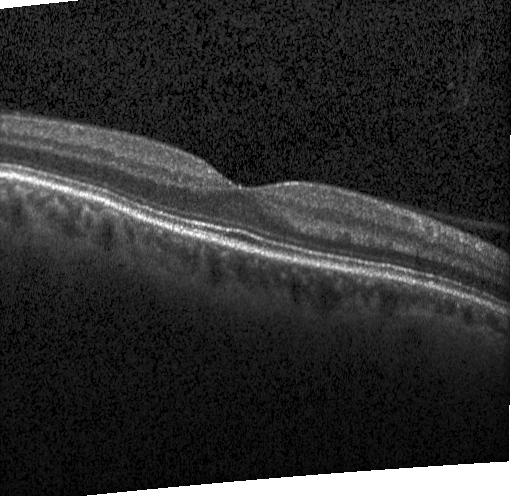

Instrument: Heidelberg Spectralis; OCT B-scan.
Macular OCT: no evidence of choroidal neovascularization, diabetic macular edema, or drusen.